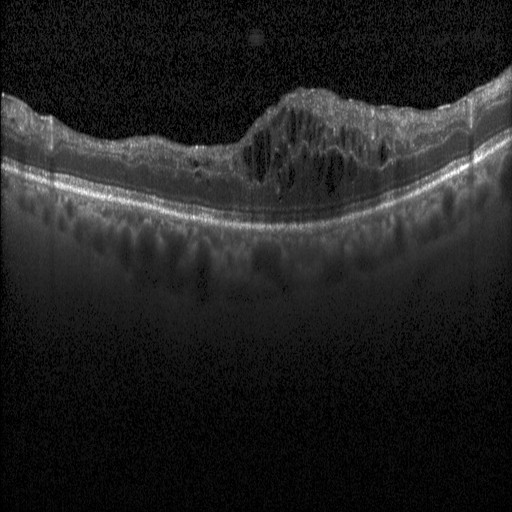 Retinal OCT cross-section, spectral-domain optical coherence tomography. Finding: diabetic macular edema (DME).